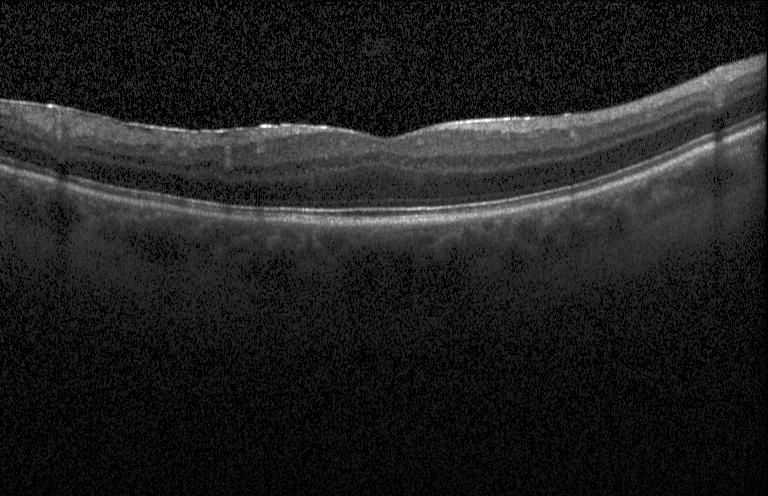 Finding: no choroidal neovascularization, no diabetic macular edema, and no drusen.